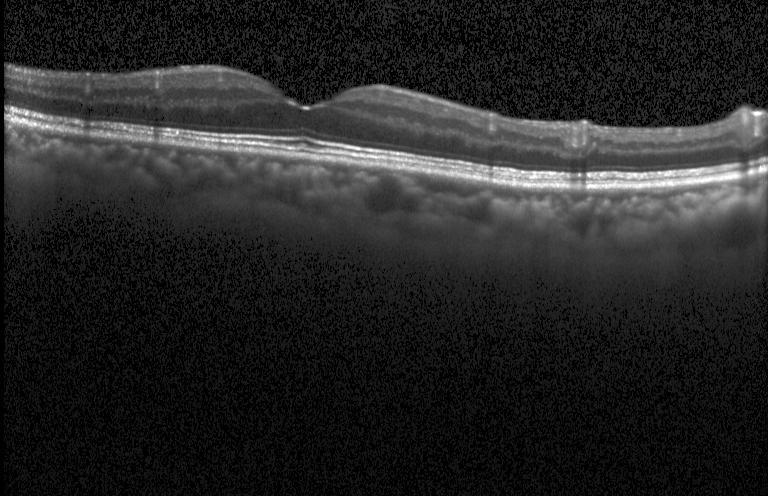

This B-scan demonstrates no choroidal neovascularization, no diabetic macular edema, and no drusen.